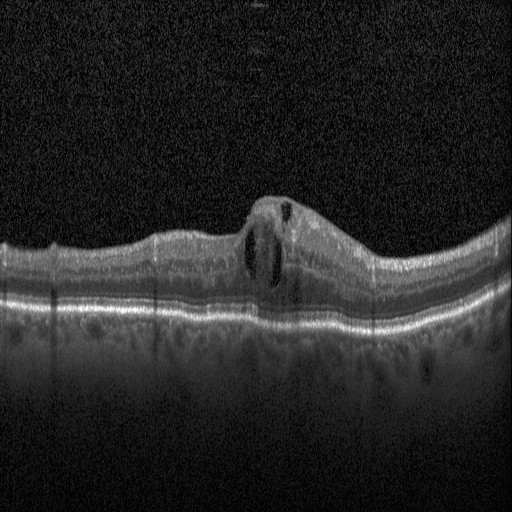

Optical coherence tomography scan · Heidelberg Spectralis · spectral-domain optical coherence tomography — Impression: diabetic macular edema (DME).